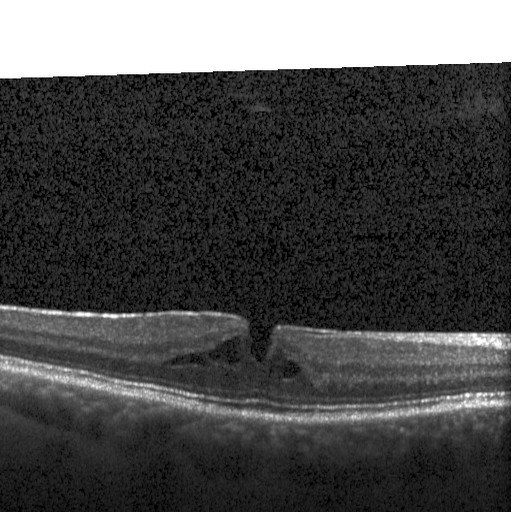
Optical coherence tomography scan
Diagnosis: diabetic macular edema (DME).